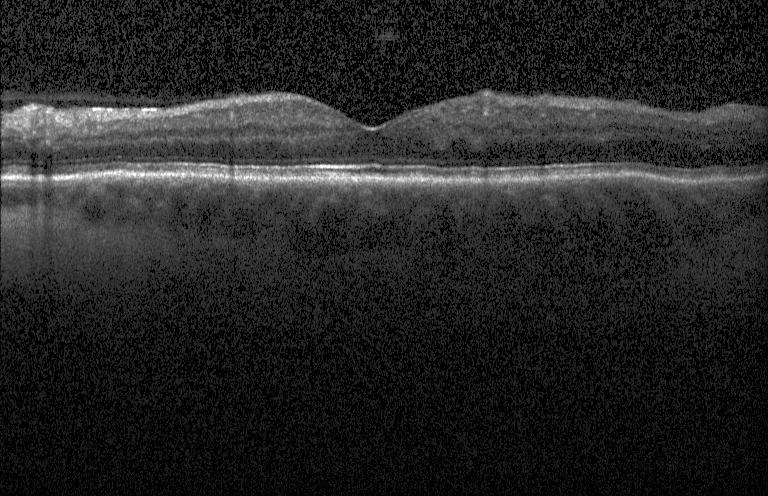 Retinal OCT B-scan · fovea-centered · spectral-domain OCT.
Diagnosis: diabetic macular edema.